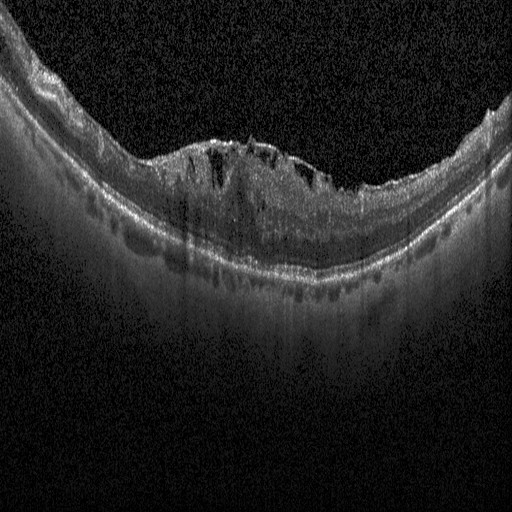 Assessment: diabetic macular edema (DME).